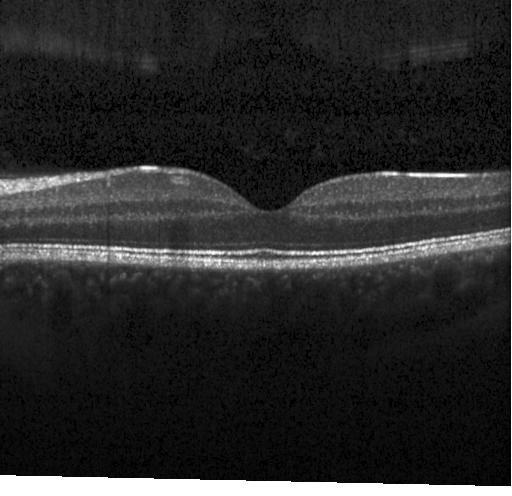

Heidelberg Spectralis, OCT B-scan, SD-OCT, macular scan
The scan shows no CNV, DME, or drusen.